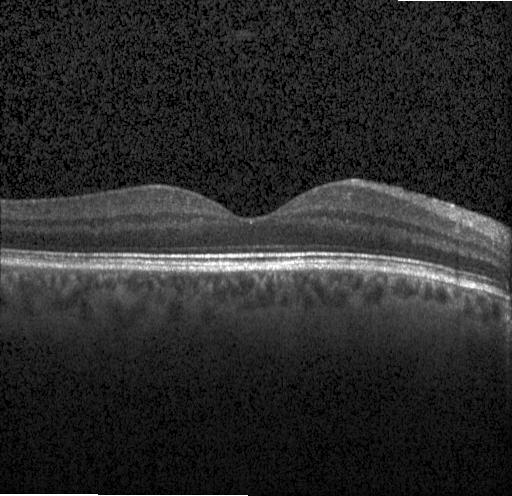 Impression: neither CNV, DME, nor drusen.